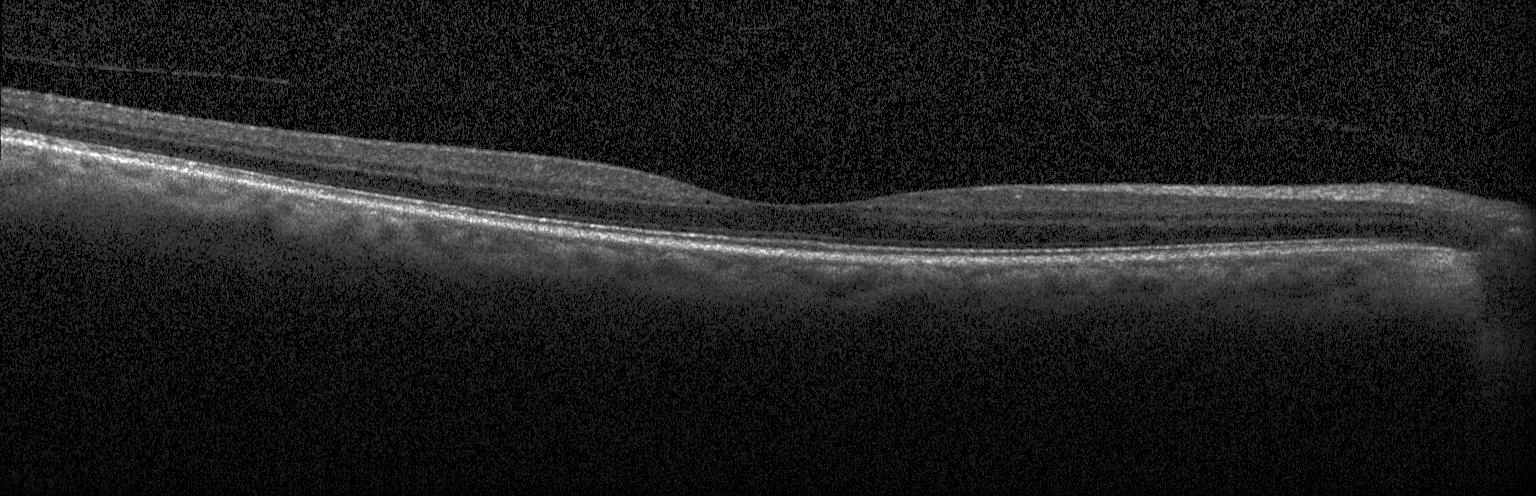 Heidelberg Spectralis OCT system; SD-OCT; optical coherence tomography B-scan; through the macula
OCT finding: no CNV, DME, or drusen.